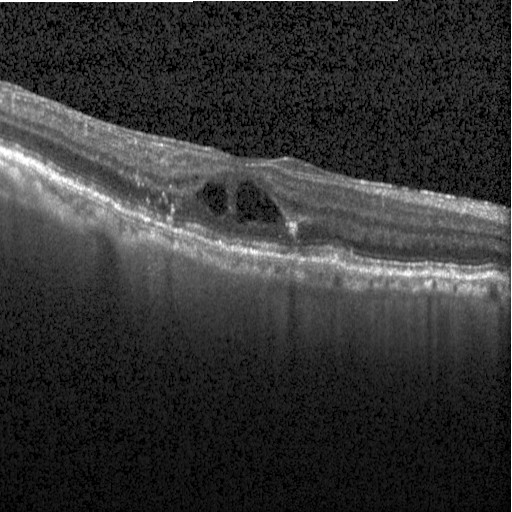
OCT B-scan, centered on the fovea — Finding: diabetic macular edema.